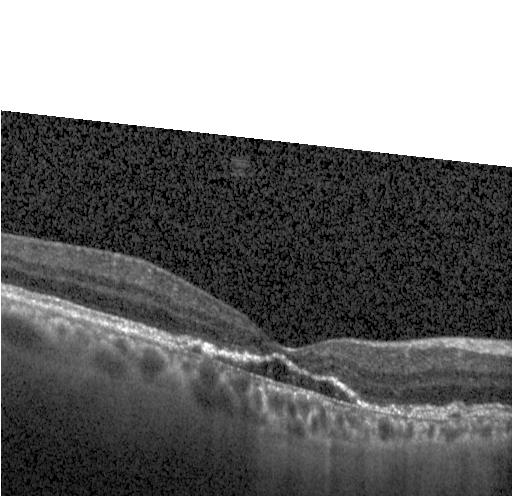

Finding: a choroidal neovascular membrane.